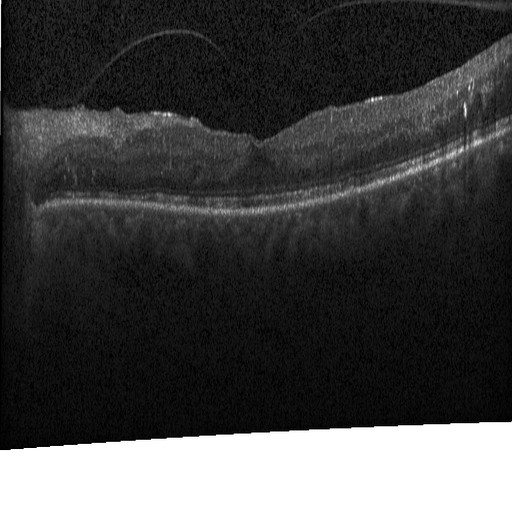 This B-scan demonstrates diabetic macular edema (DME).